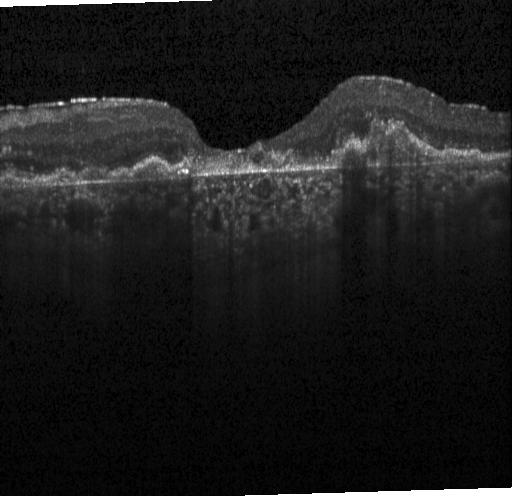

OCT scan showing CNV.